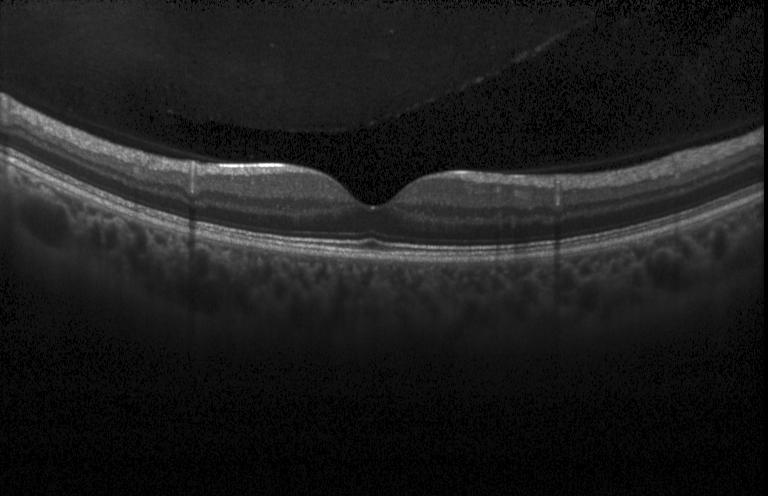 Retinal OCT B-scan; Heidelberg Spectralis OCT system; horizontal scan through the fovea
Diagnosis: no choroidal neovascularization, no diabetic macular edema, and no drusen.